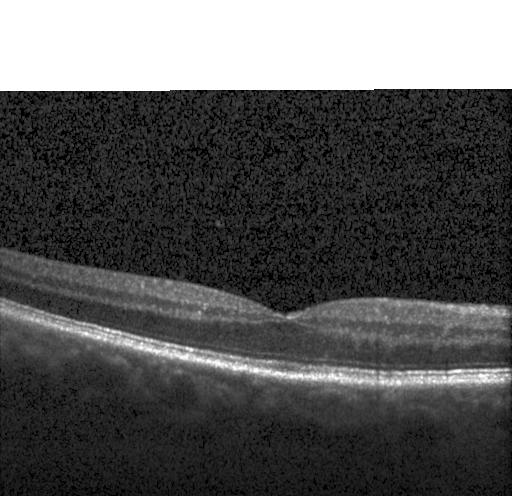
OCT B-scan
Impression: no CNV, DME, or drusen.